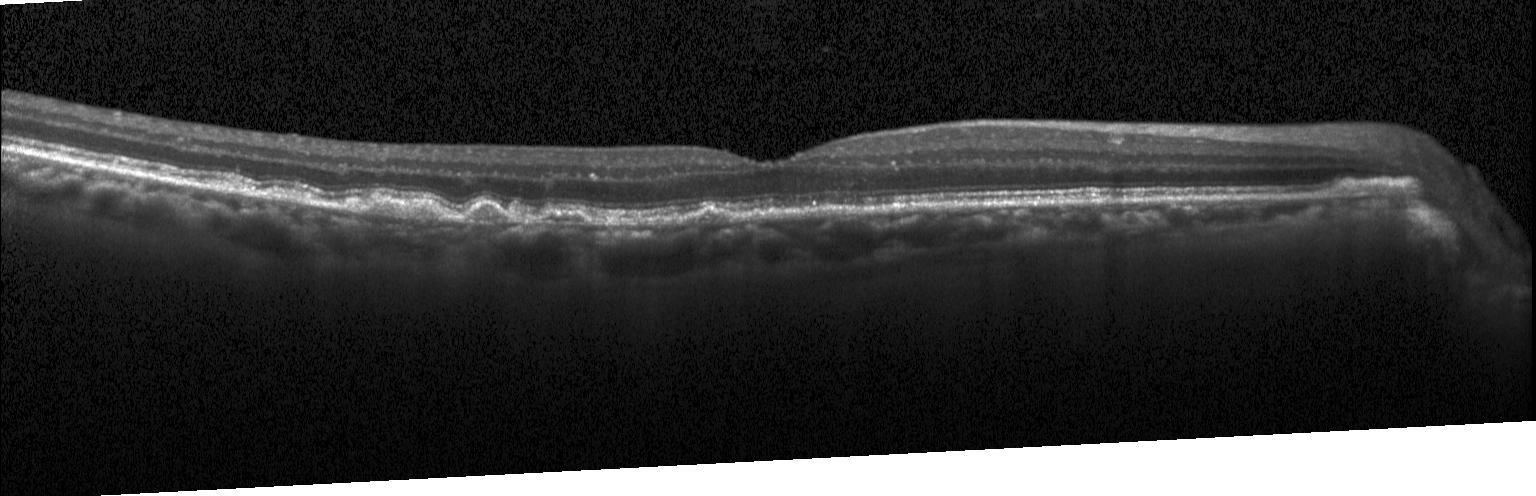 Optical coherence tomography scan
Macular OCT: multiple drusen.